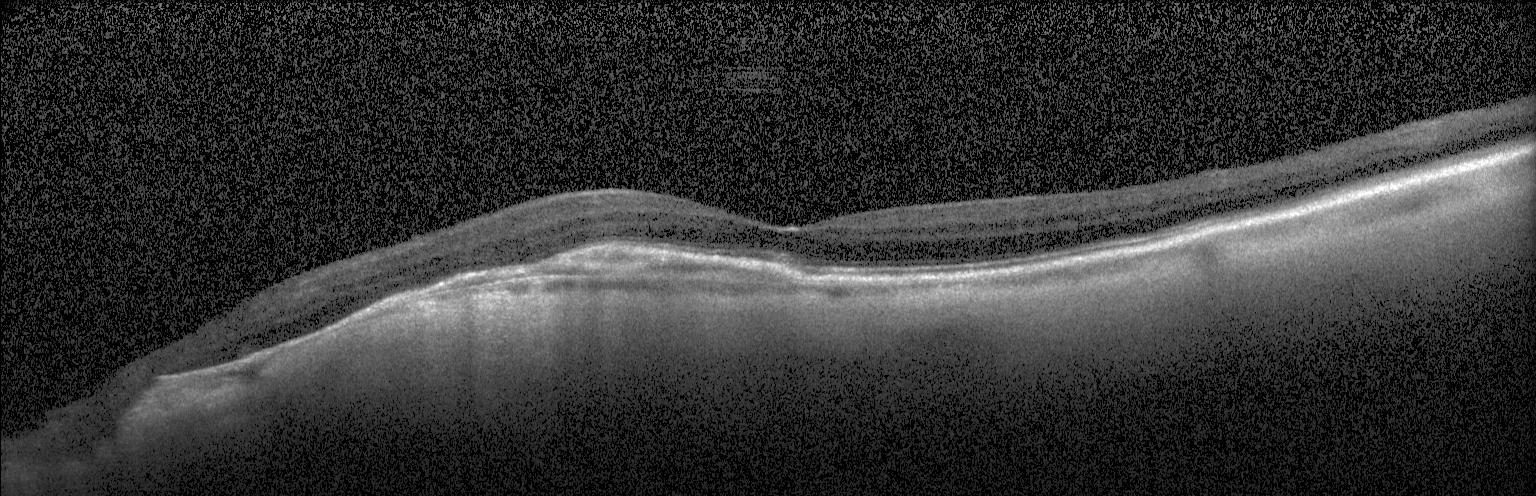

OCT line scan — Macular OCT: a choroidal neovascular membrane.